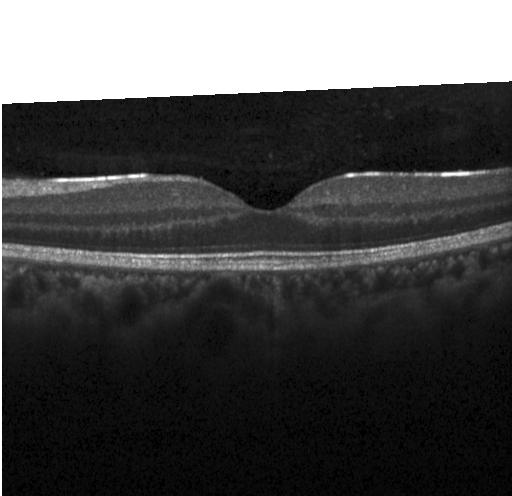

Spectral-domain OCT · Heidelberg Spectralis OCT system · OCT B-scan · centered on the fovea. Impression: no choroidal neovascularization, no diabetic macular edema, and no drusen.